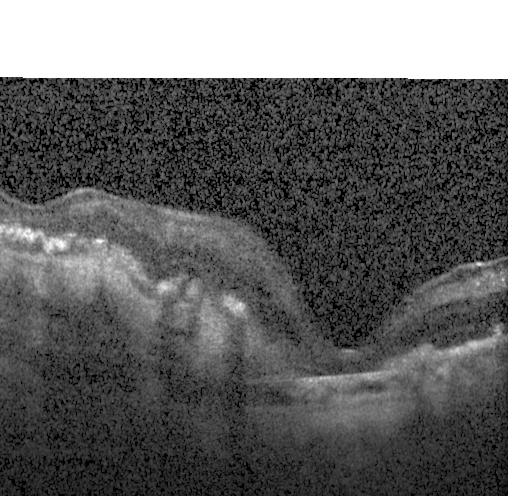

Retinal OCT B-scan — OCT finding: choroidal neovascularization (CNV).